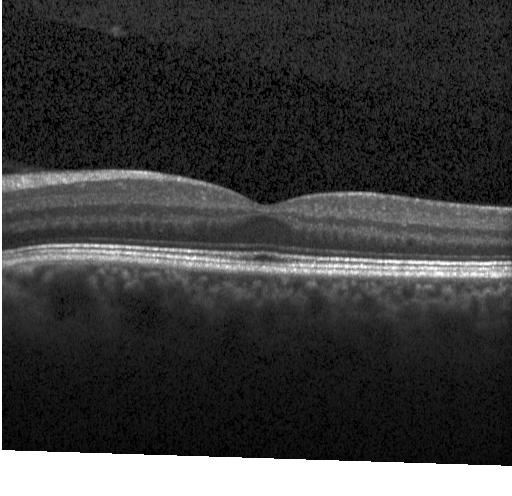

Optical coherence tomography scan.
Impression: neither CNV, DME, nor drusen.